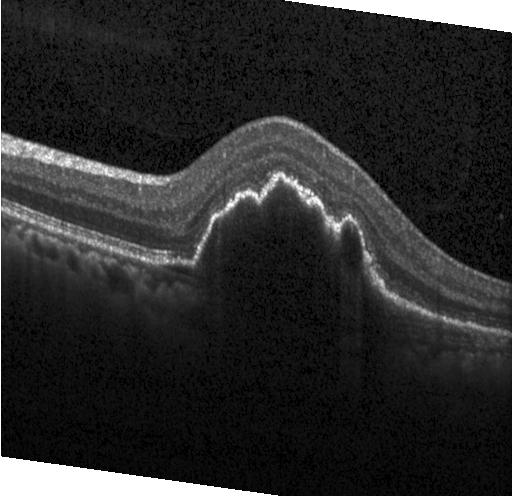 Through the macula; SD-OCT; optical coherence tomography scan; acquired on a Heidelberg Spectralis.
Diagnosis: CNV.